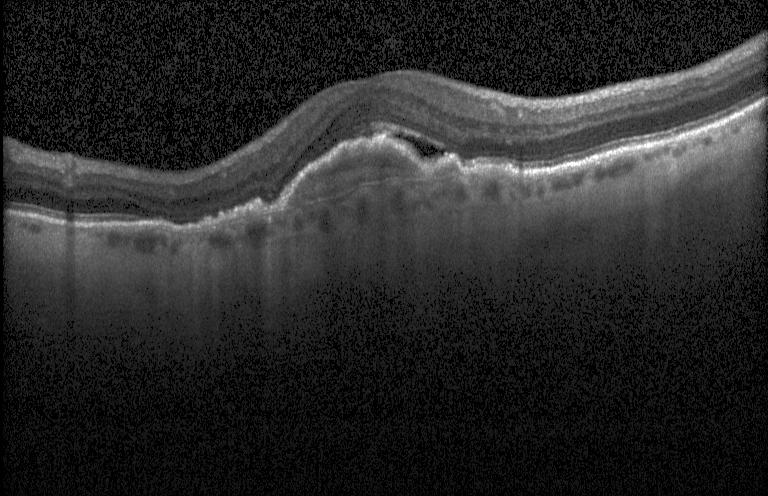

Impression: choroidal neovascularization (CNV).